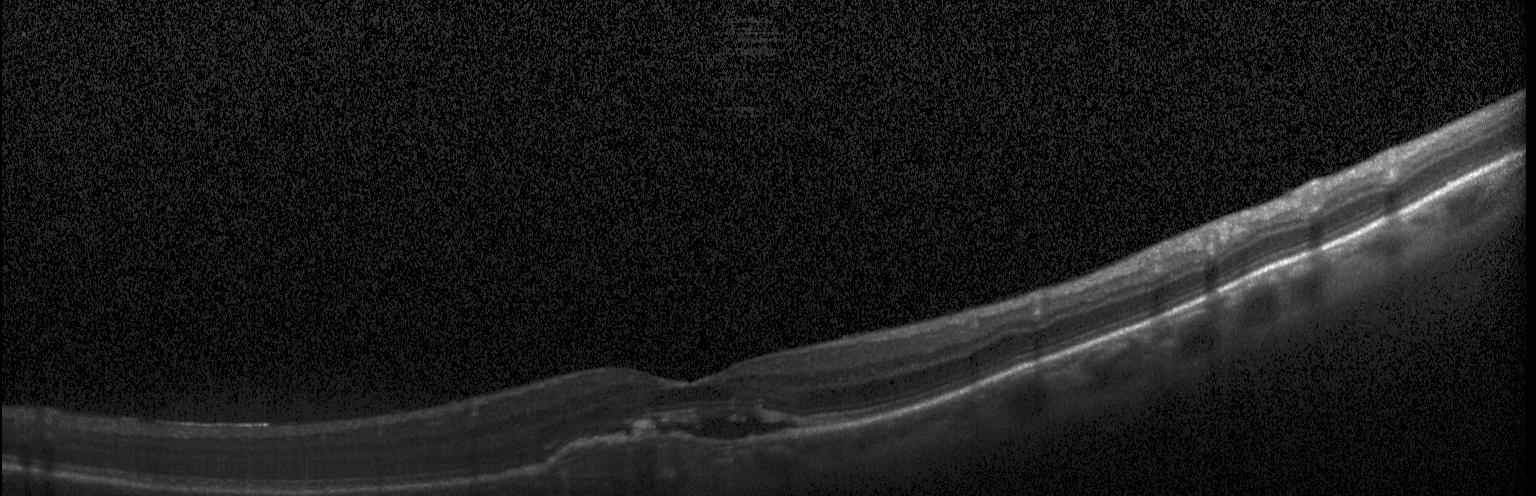 Dx: CNV.